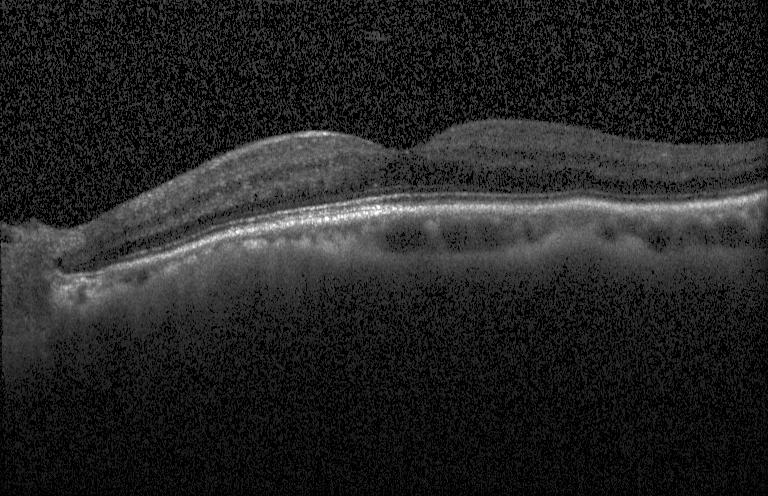

Heidelberg Spectralis OCT system, retinal OCT cross-section. Macular OCT: no CNV, no DME, and no drusen.